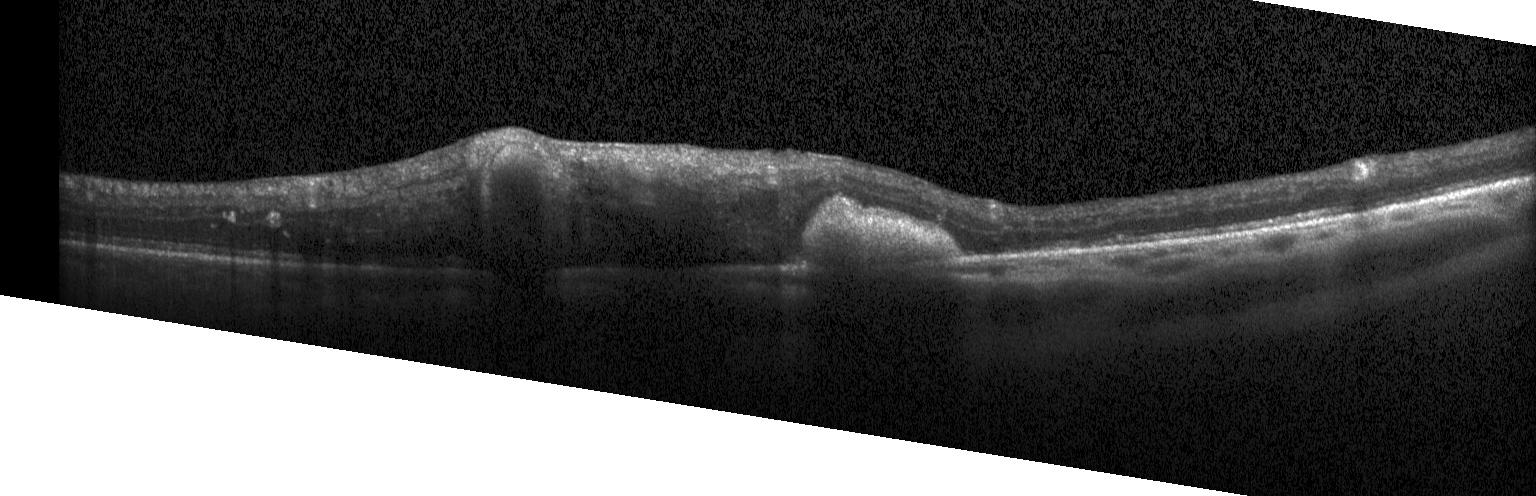

Retinal OCT B-scan. This B-scan demonstrates choroidal neovascularization.